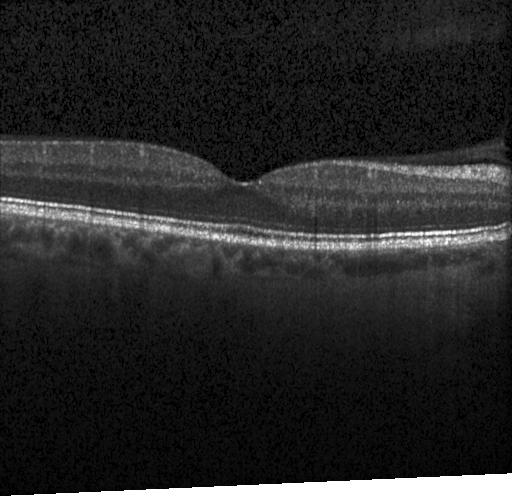 OCT B-scan · through the macula · spectral-domain OCT.
Diagnosis: no CNV, DME, or drusen.